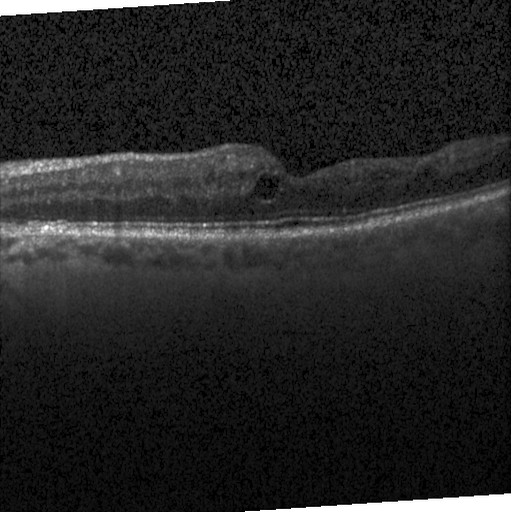

Retinal OCT B-scan · spectral-domain optical coherence tomography. Impression: diabetic macular edema.